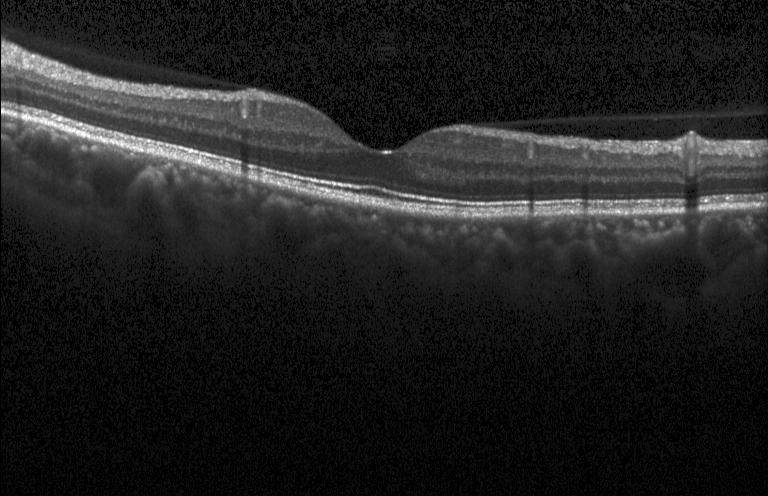

OCT B-scan — Impression: no evidence of choroidal neovascularization, diabetic macular edema, or drusen.